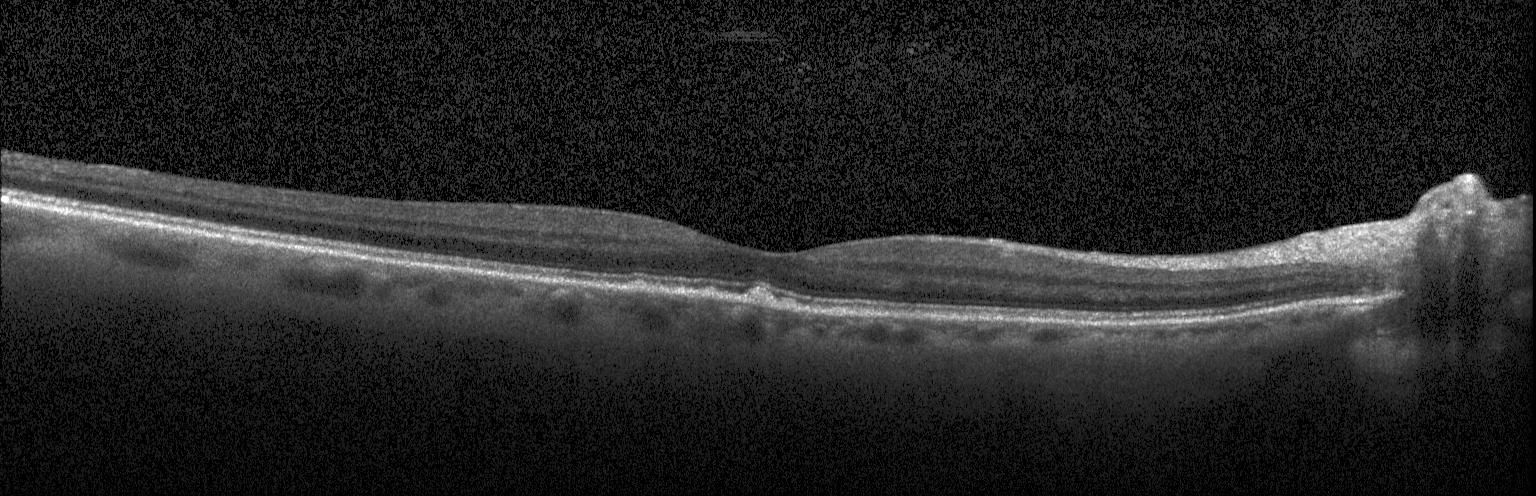
OCT line scan — Assessment: drusen.